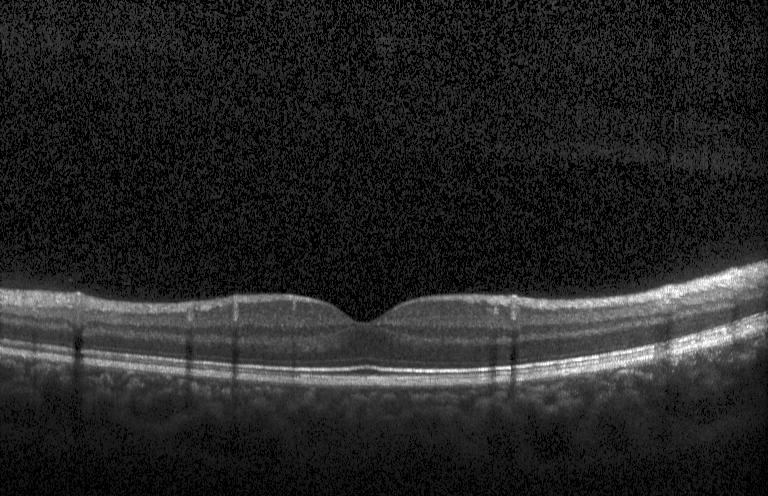
Macular OCT: no evidence of CNV, DME, or drusen.